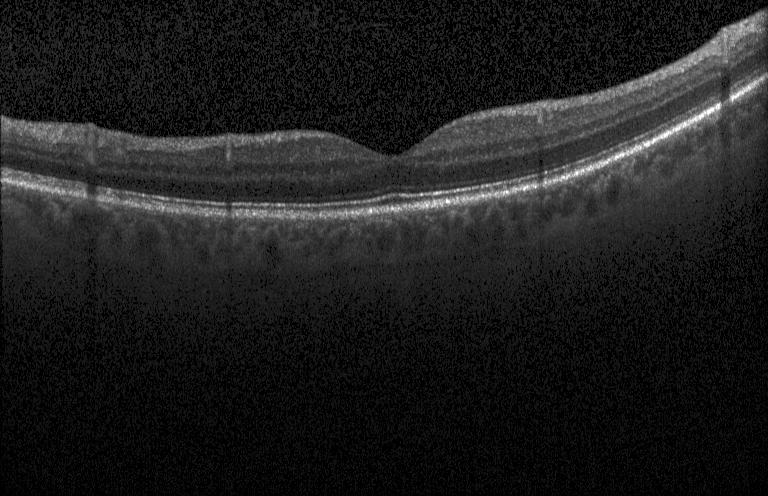
Horizontal scan through the fovea. Optical coherence tomography scan — No evidence of choroidal neovascularization, diabetic macular edema, or drusen.